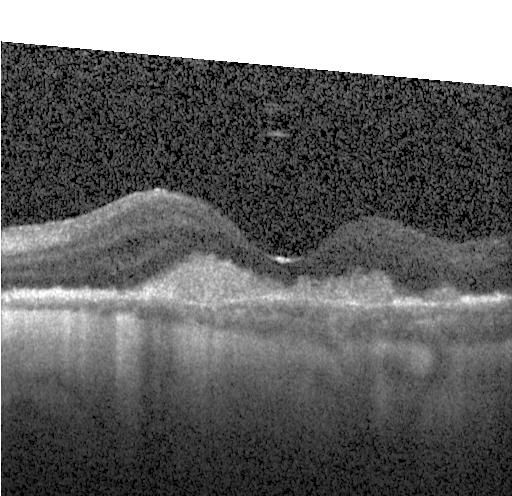
Centered on the fovea. Optical coherence tomography scan. Spectral-domain optical coherence tomography.
Finding: a choroidal neovascular membrane.